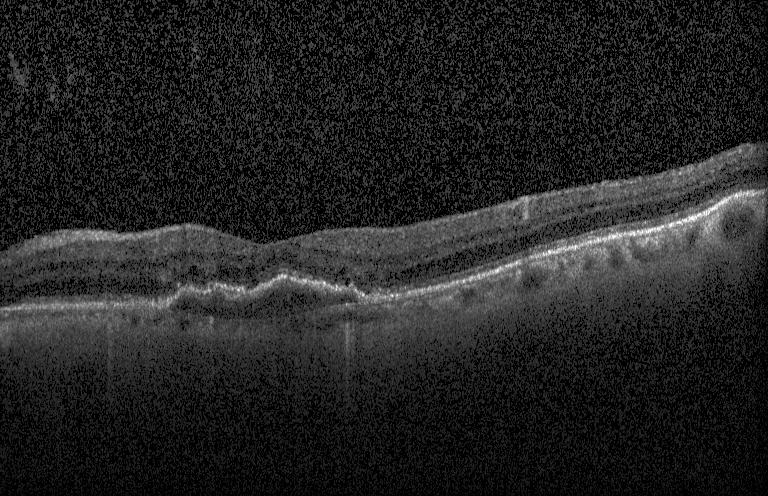
Impression: choroidal neovascularization (CNV).